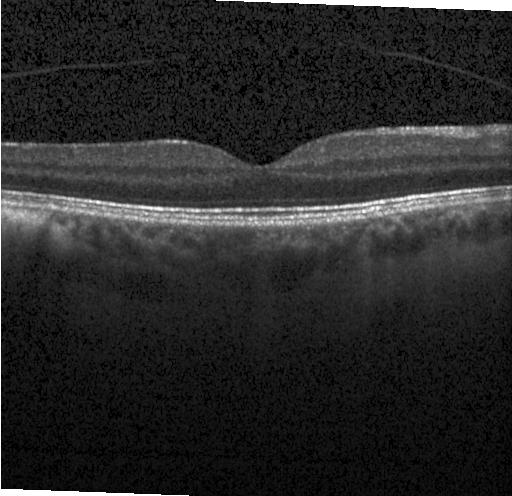
Macular scan, acquired on a Heidelberg Spectralis, spectral-domain optical coherence tomography, retinal OCT cross-section
Finding: no CNV, no DME, and no drusen.